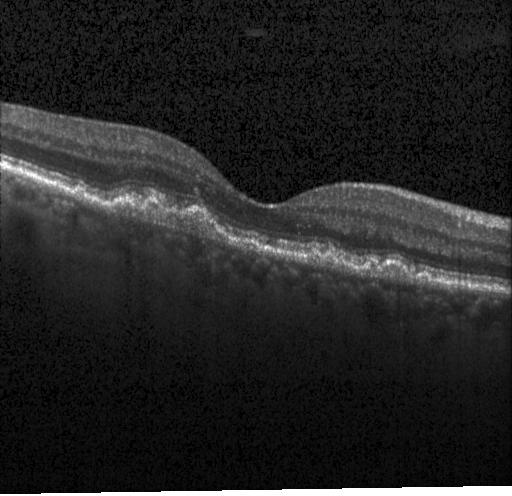

OCT B-scan.
Dx: a choroidal neovascular membrane.